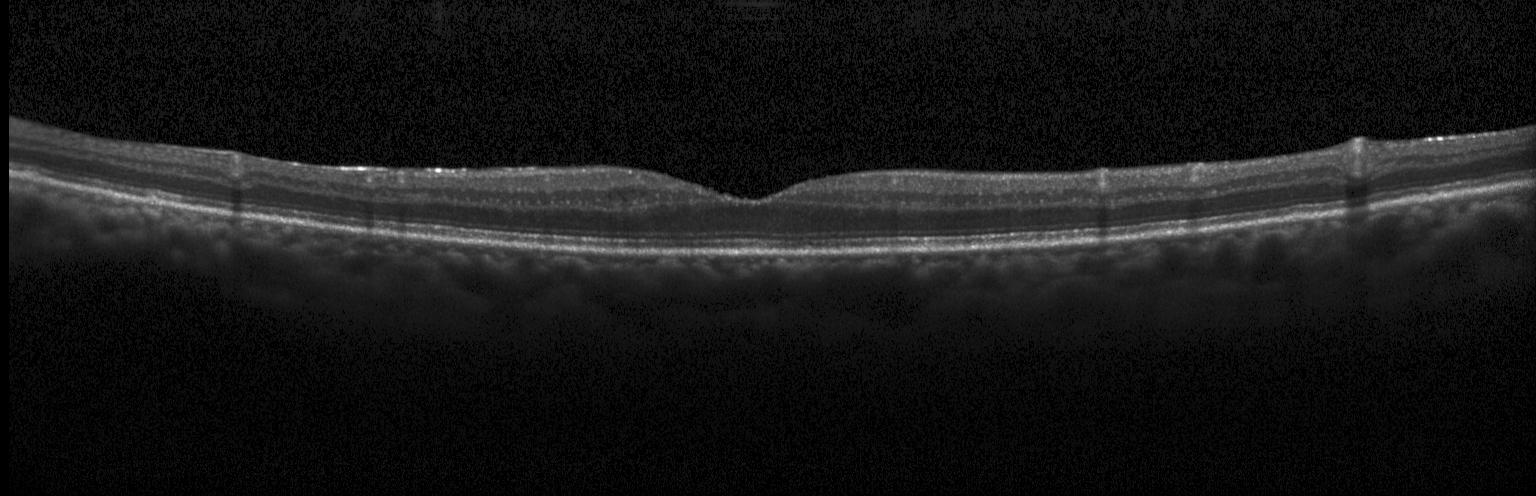

OCT scan showing neither CNV, DME, nor drusen.